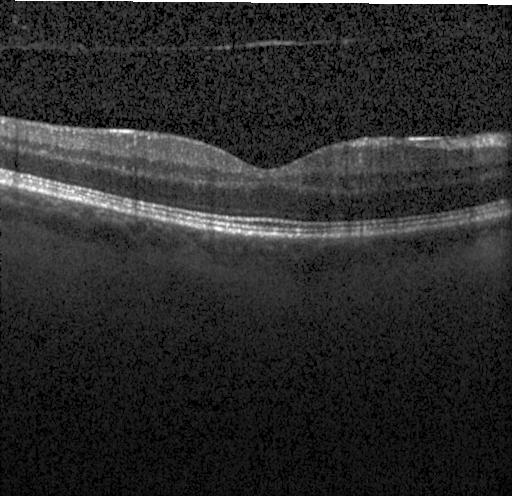

Retinal OCT cross-section.
This B-scan demonstrates neither choroidal neovascularization, diabetic macular edema, nor drusen.